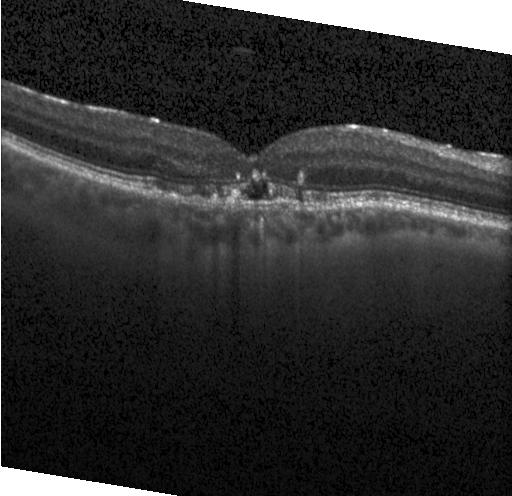 Assessment: a choroidal neovascular membrane.